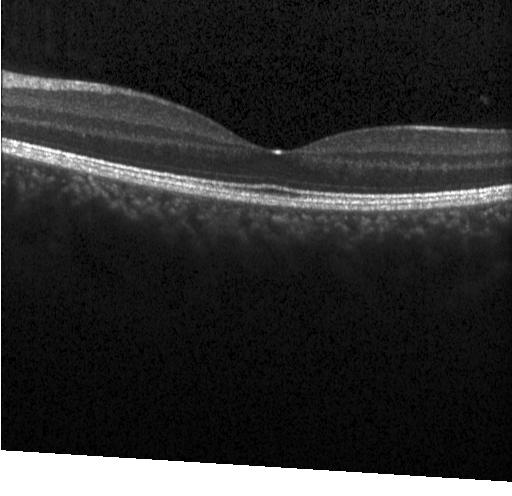

SD-OCT, OCT line scan, Heidelberg Spectralis, horizontal scan through the fovea.
Finding: no choroidal neovascularization, no diabetic macular edema, and no drusen.